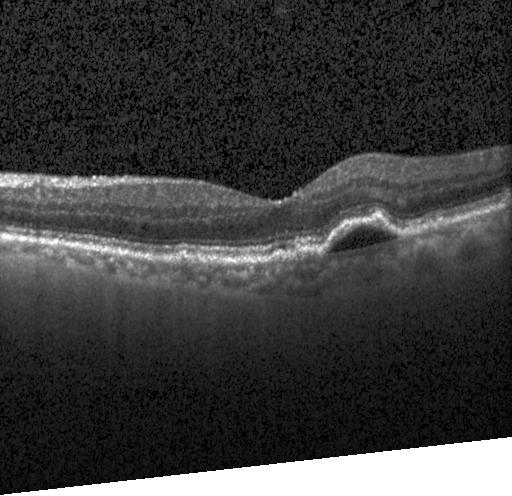
Diagnosis: a choroidal neovascular membrane.